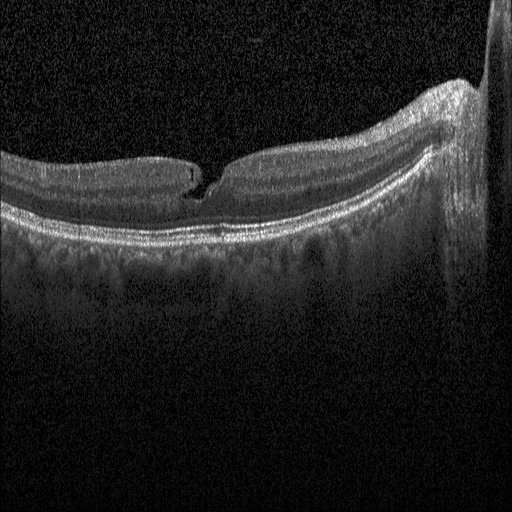

Diagnosis: diabetic macular edema (DME).